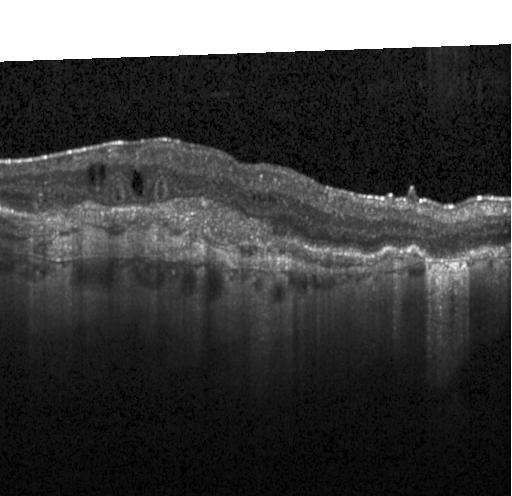
Finding: a choroidal neovascular membrane.